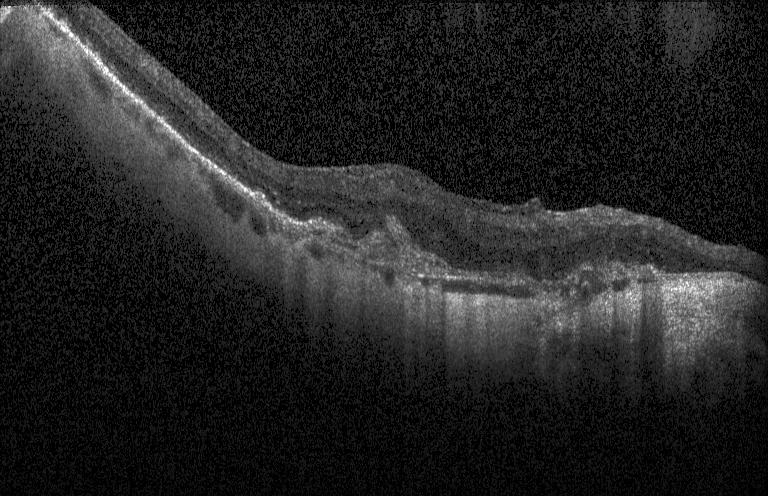
Retinal OCT B-scan, centered on the fovea. The scan shows a choroidal neovascular membrane.